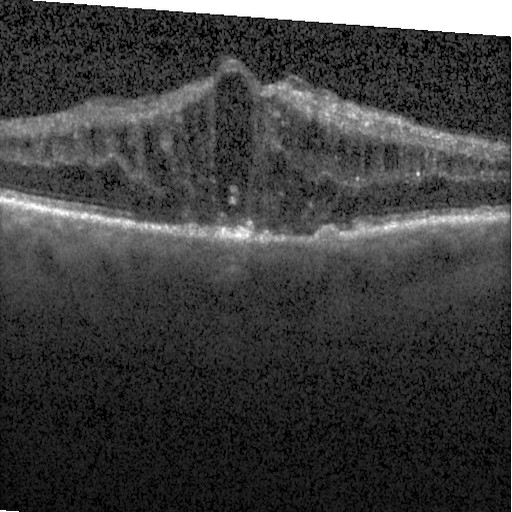 Retinal OCT B-scan, macular scan — Diagnosis: diabetic macular edema (DME).